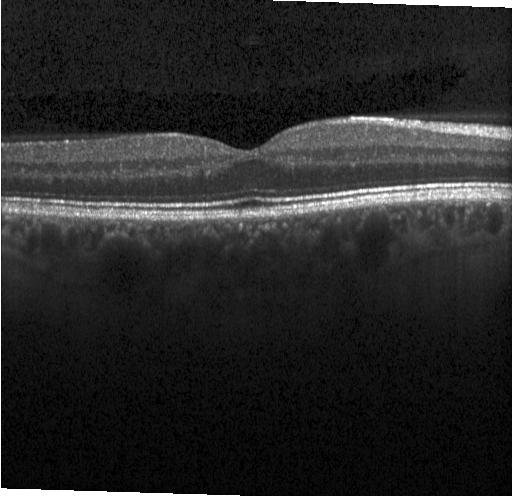 The scan shows no CNV, no DME, and no drusen.